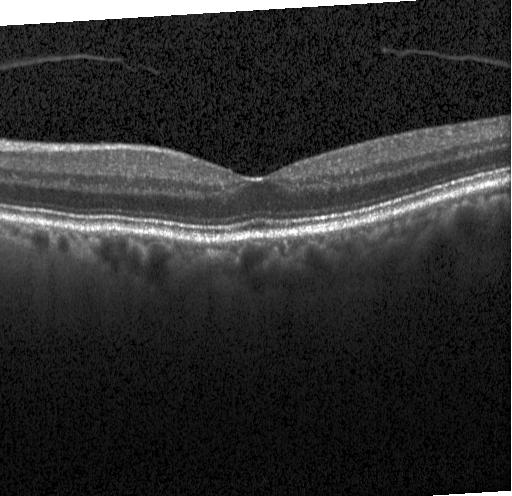

Macular scan, retinal OCT cross-section, SD-OCT, Heidelberg Spectralis OCT system — Dx: no choroidal neovascularization, diabetic macular edema, or drusen.